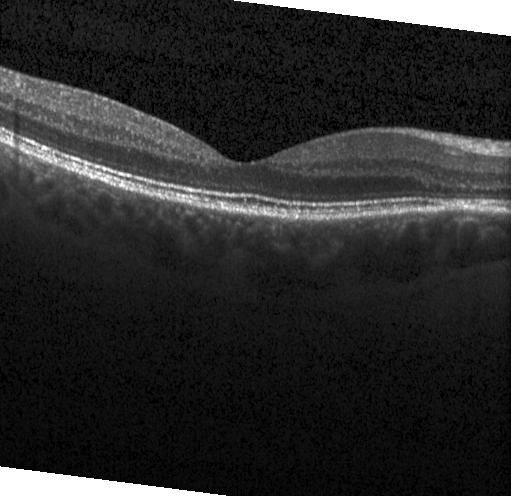
Retinal OCT cross-section; spectral-domain OCT; Heidelberg Spectralis; through the macula. Impression: no evidence of choroidal neovascularization, diabetic macular edema, or drusen.